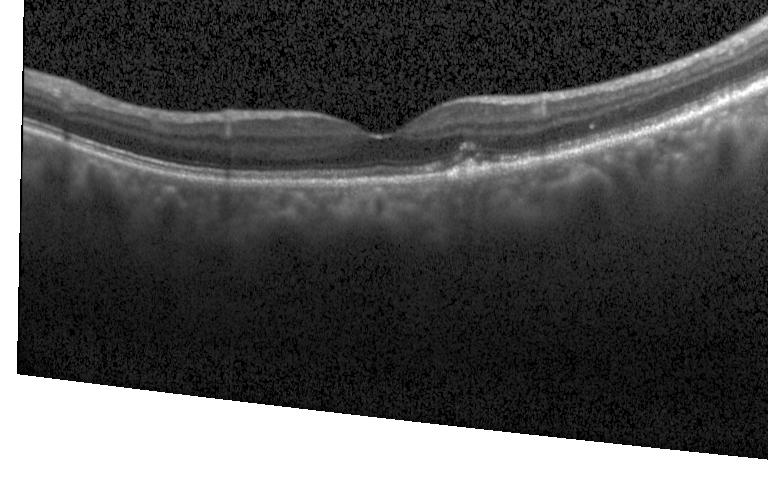
Centered on the fovea, optical coherence tomography B-scan. Sub-RPE drusenoid deposits.